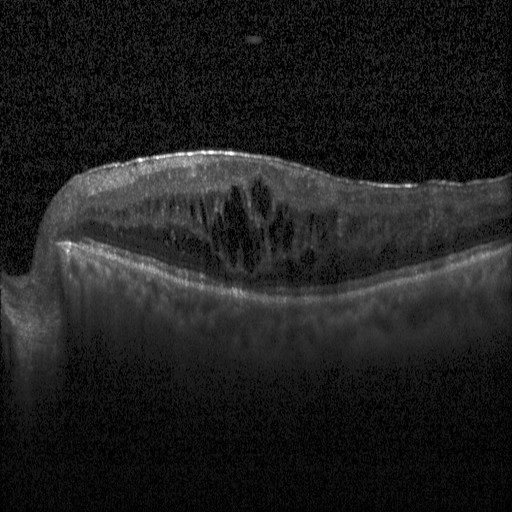
OCT B-scan — Diagnosis: diabetic macular edema.